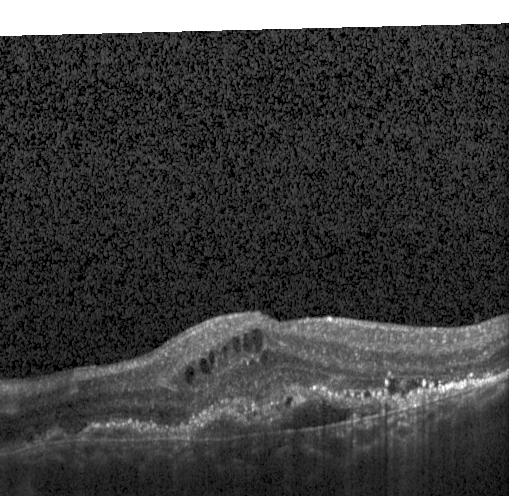 Optical coherence tomography B-scan. OCT finding: a choroidal neovascular membrane.